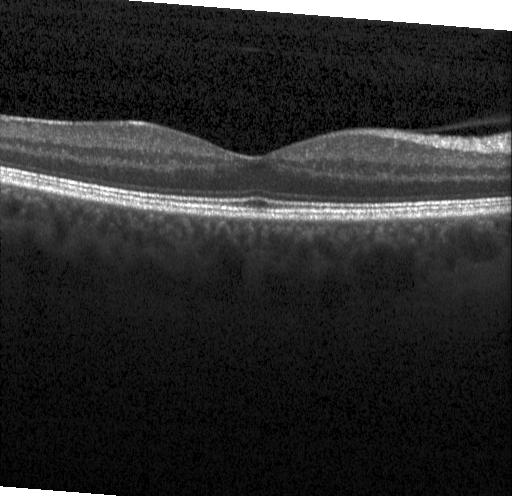 Retinal OCT B-scan · spectral-domain OCT — Neither CNV, DME, nor drusen.